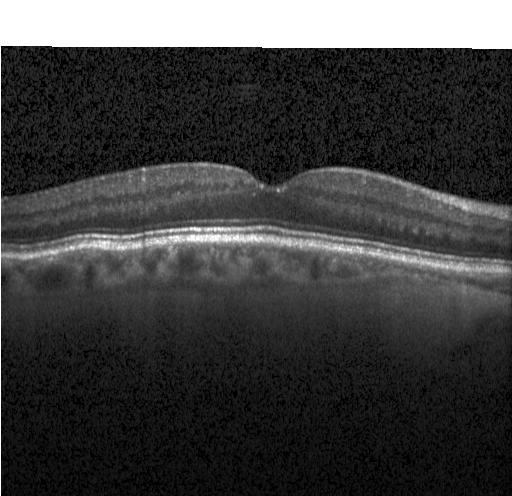

OCT line scan, fovea-centered, acquired on a Heidelberg Spectralis — Dx: no choroidal neovascularization, diabetic macular edema, or drusen.